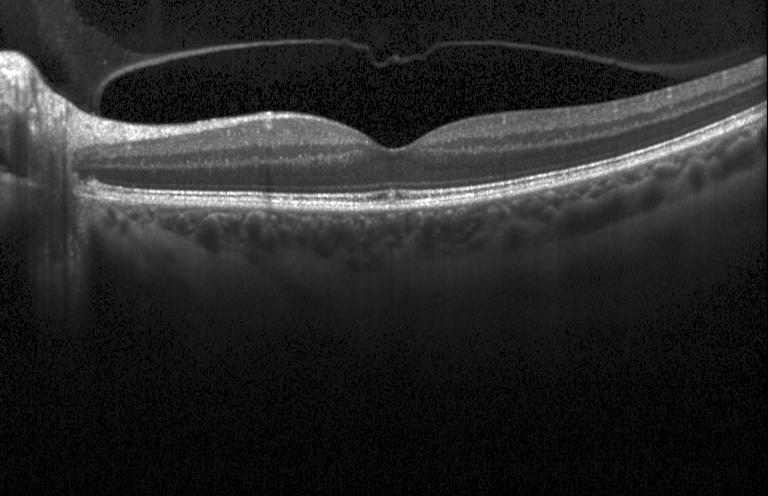 Spectral-domain OCT B-scan: no choroidal neovascularization, diabetic macular edema, or drusen.